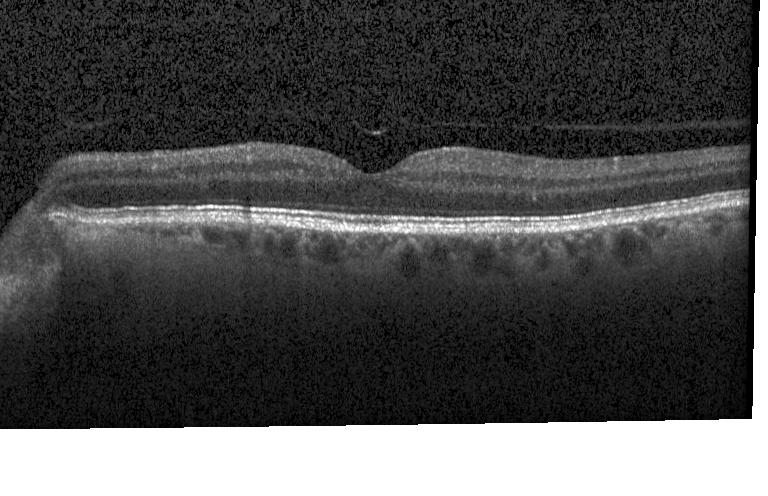
Retinal OCT cross-section, spectral-domain OCT, Heidelberg Spectralis OCT system
Dx: no evidence of CNV, DME, or drusen.